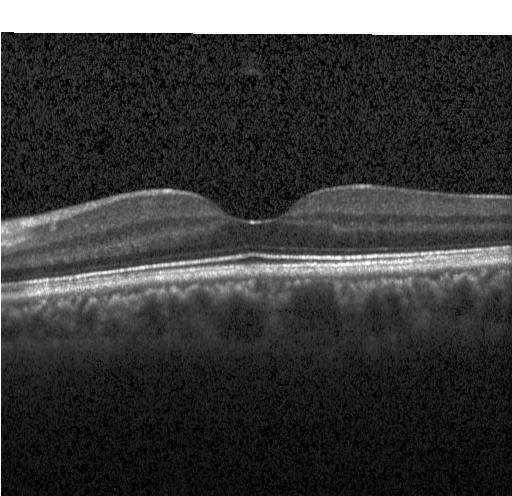

Retinal OCT B-scan
Assessment: no choroidal neovascularization, diabetic macular edema, or drusen.